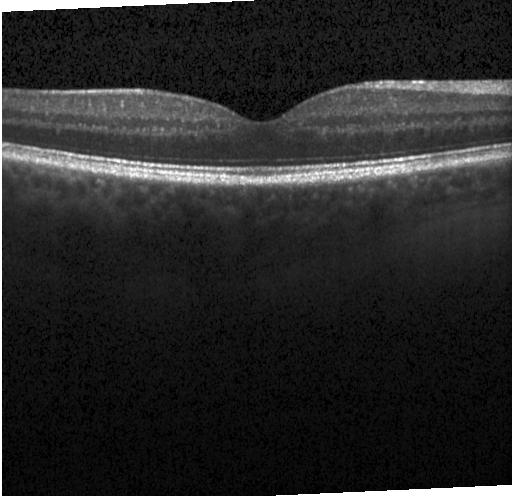 Macular OCT: neither choroidal neovascularization, diabetic macular edema, nor drusen.